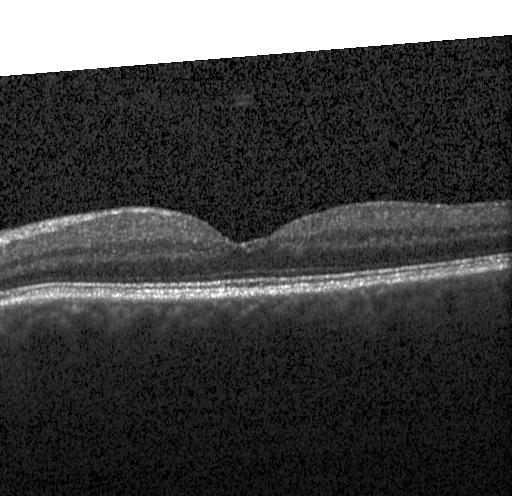
Horizontal scan through the fovea, OCT B-scan, spectral-domain OCT
Impression: no evidence of choroidal neovascularization, diabetic macular edema, or drusen.